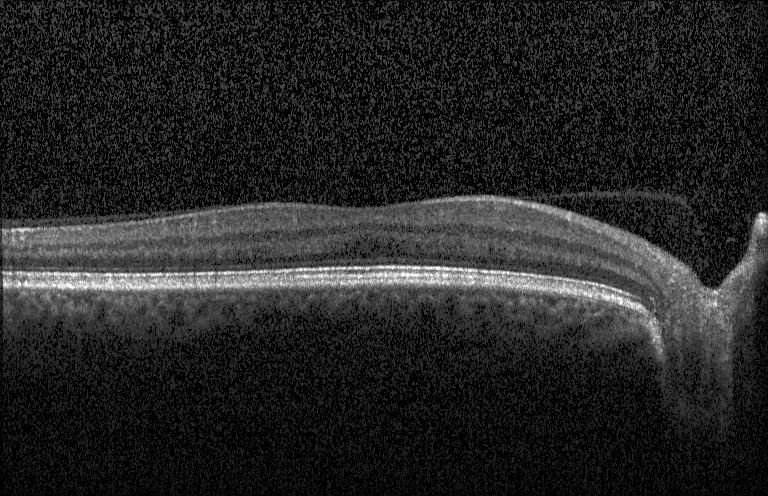
SD-OCT. Acquired on a Heidelberg Spectralis. OCT line scan. Through the macula.
Impression: no evidence of choroidal neovascularization, diabetic macular edema, or drusen.